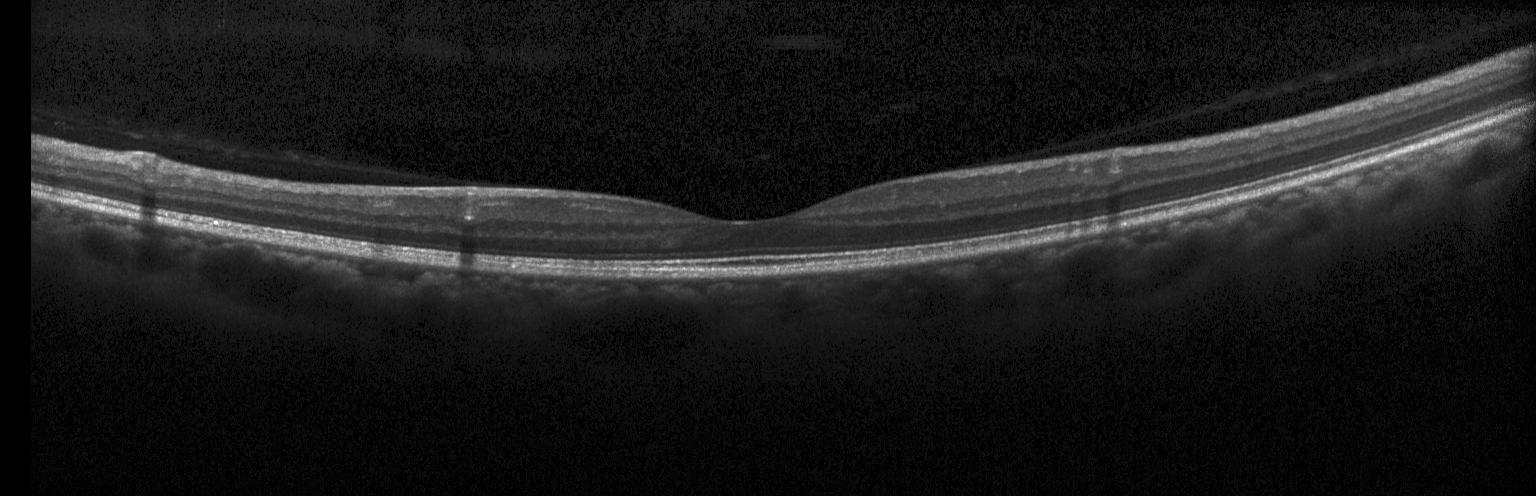 Macular OCT demonstrating neither choroidal neovascularization, diabetic macular edema, nor drusen.